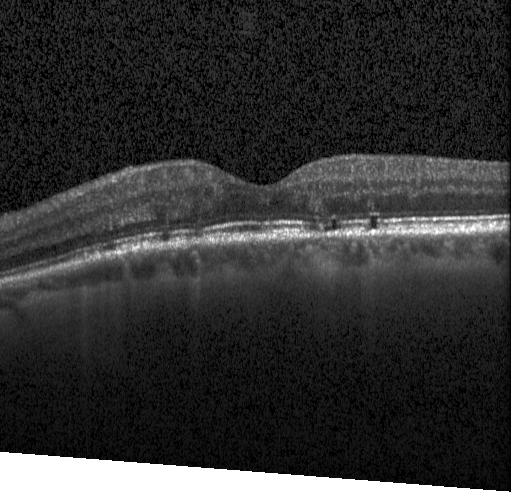 OCT scan showing diabetic macular edema (DME).